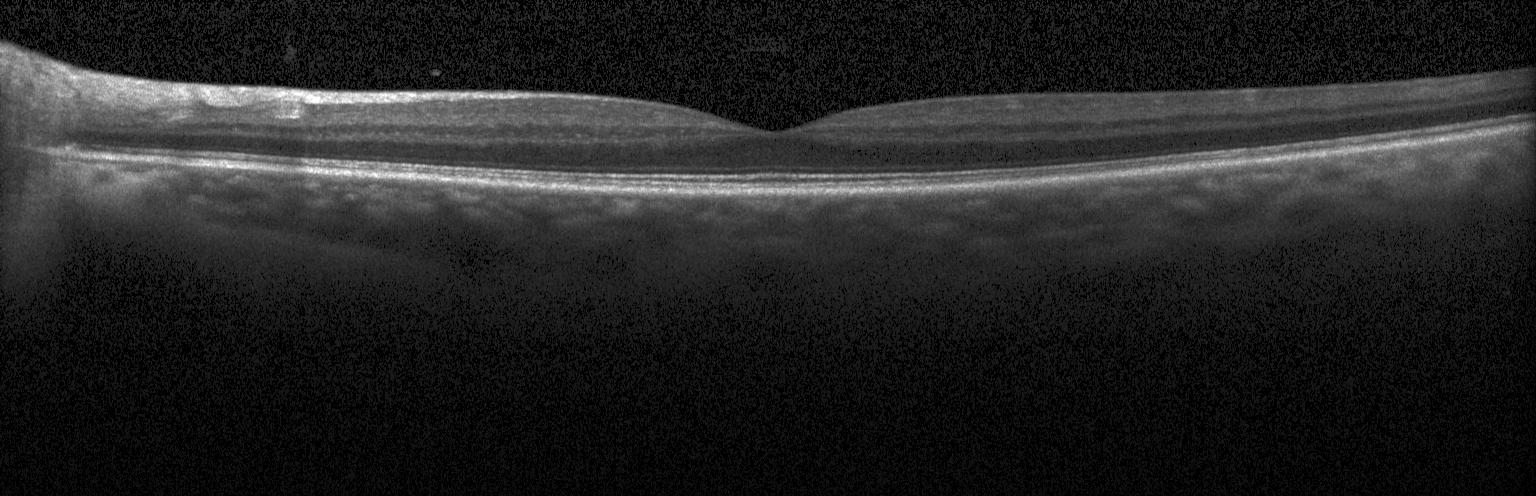
SD-OCT · optical coherence tomography B-scan · centered on the fovea — Dx: neither CNV, DME, nor drusen.